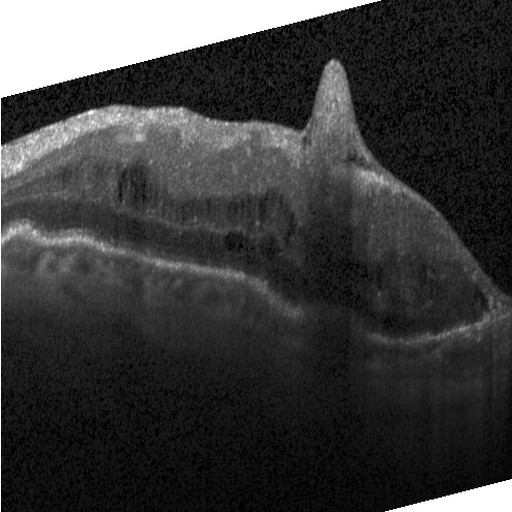 Spectral-domain optical coherence tomography. Retinal OCT B-scan. Centered on the fovea. Heidelberg Spectralis OCT system — Diagnosis: diabetic macular edema.